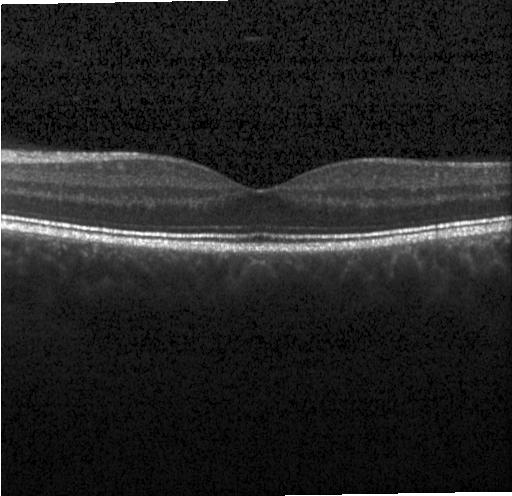
SD-OCT. Optical coherence tomography B-scan. Heidelberg Spectralis. Centered on the fovea. The scan shows no evidence of choroidal neovascularization, diabetic macular edema, or drusen.